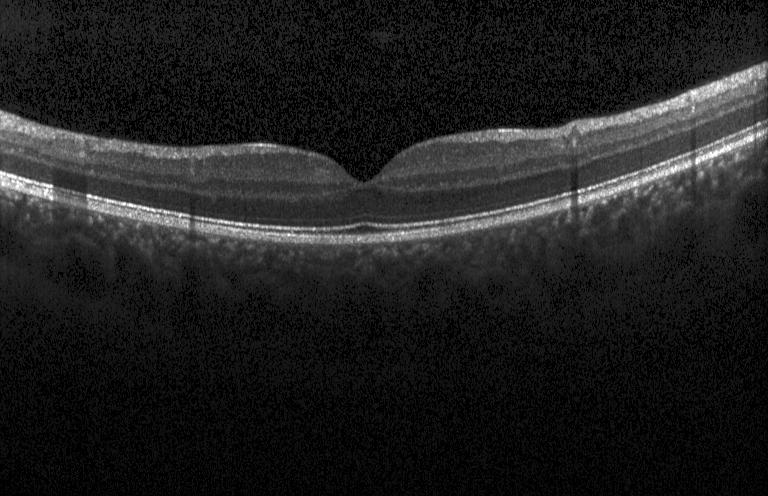
Retinal OCT cross-section showing no CNV, DME, or drusen.